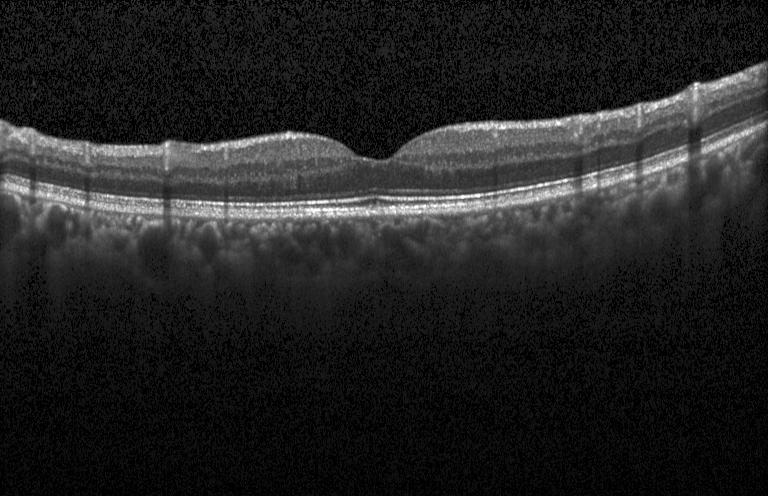
Instrument: Heidelberg Spectralis; optical coherence tomography B-scan; centered on the fovea.
This B-scan demonstrates neither choroidal neovascularization, diabetic macular edema, nor drusen.